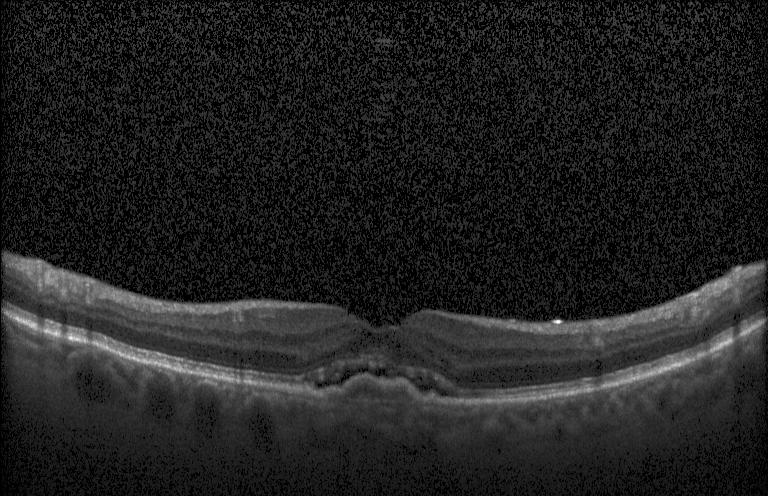

Through the macula, Heidelberg Spectralis OCT system, OCT B-scan, spectral-domain optical coherence tomography.
Impression: choroidal neovascularization.